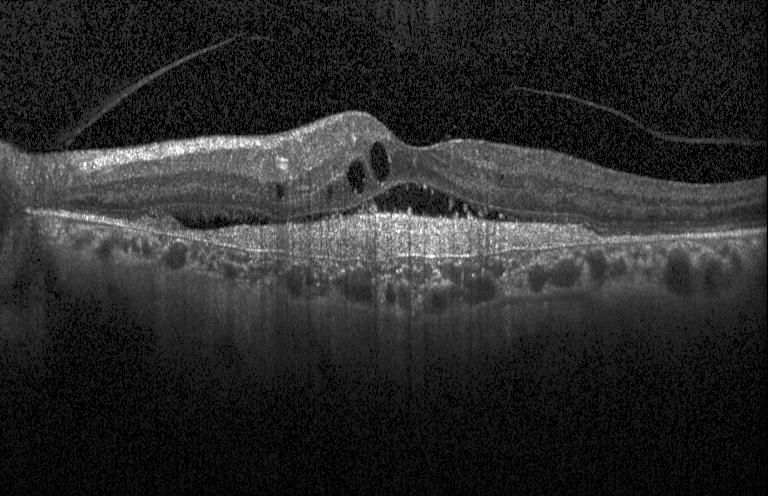 Retinal OCT cross-section
Finding: a choroidal neovascular membrane.